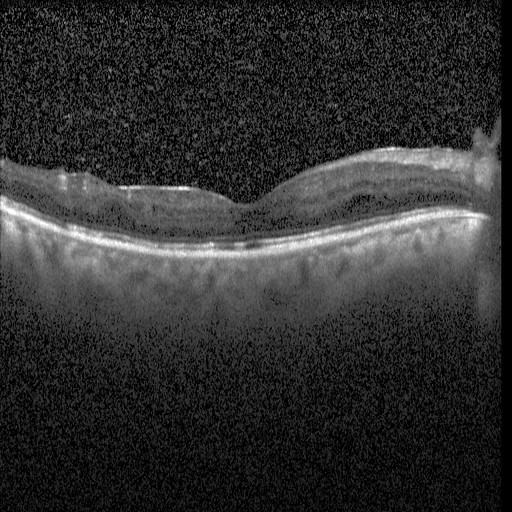

OCT B-scan showing DME.